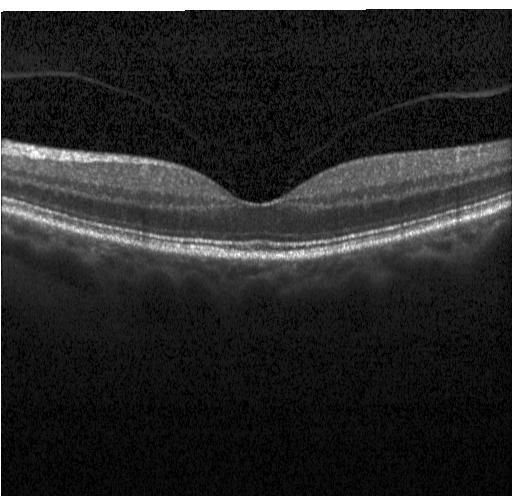 Impression: no evidence of choroidal neovascularization, diabetic macular edema, or drusen.